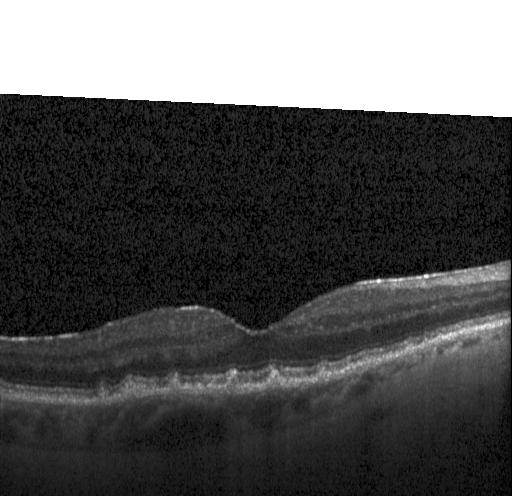 Instrument: Heidelberg Spectralis; optical coherence tomography scan — This B-scan demonstrates drusen.